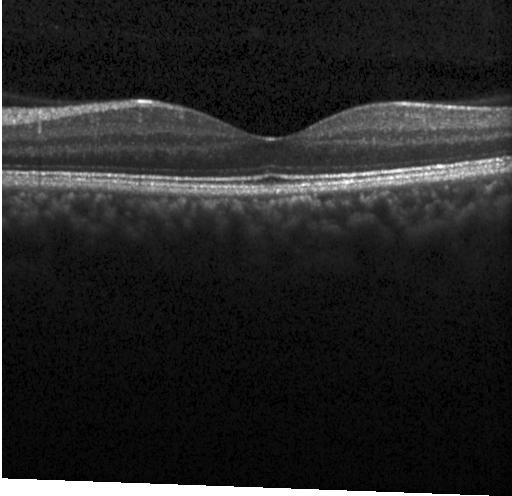 Diagnosis: no choroidal neovascularization, no diabetic macular edema, and no drusen.